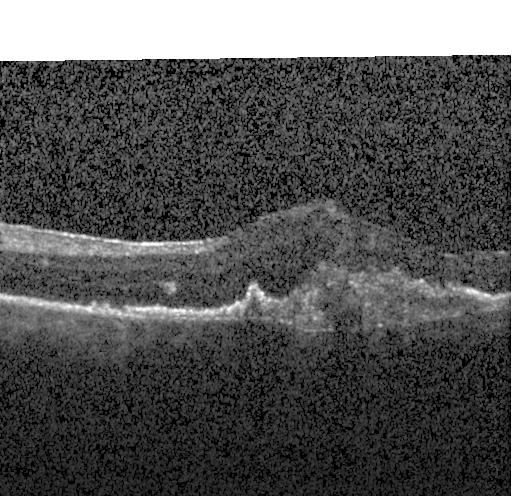
Optical coherence tomography B-scan; instrument: Heidelberg Spectralis; horizontal scan through the fovea. Dx: a choroidal neovascular membrane.